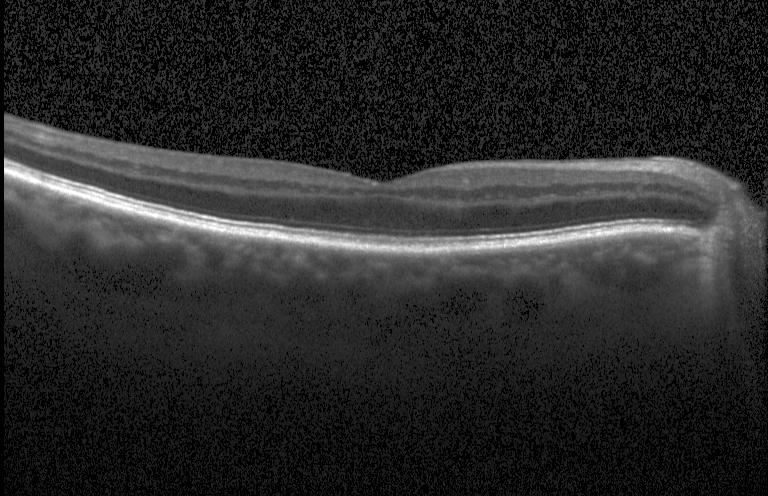
Spectral-domain optical coherence tomography, acquired on a Heidelberg Spectralis, retinal OCT B-scan, horizontal scan through the fovea
Macular OCT: no evidence of choroidal neovascularization, diabetic macular edema, or drusen.